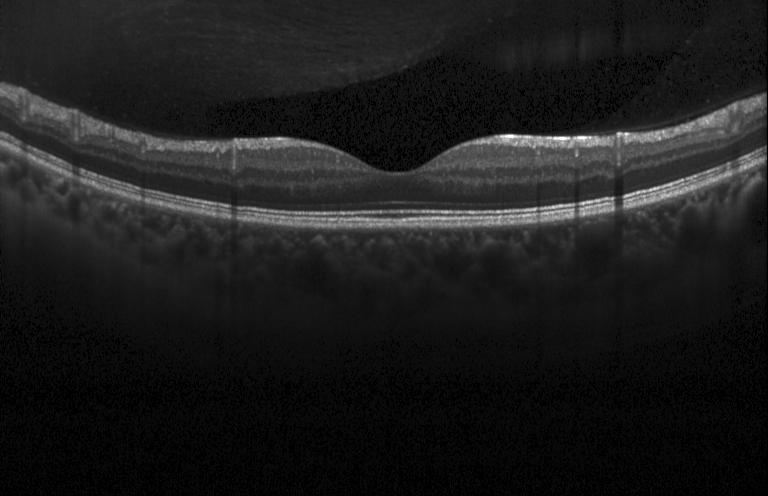
Retinal OCT cross-section
Finding: no evidence of choroidal neovascularization, diabetic macular edema, or drusen.